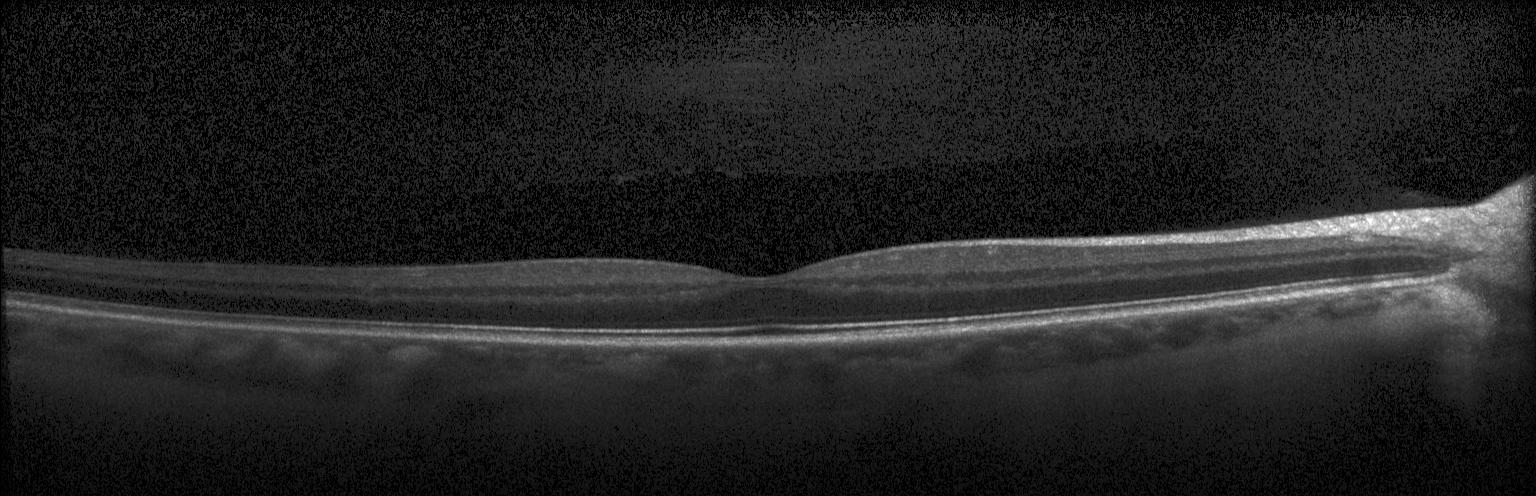

Retinal OCT cross-section, instrument: Heidelberg Spectralis, through the macula.
The scan shows no choroidal neovascularization, no diabetic macular edema, and no drusen.